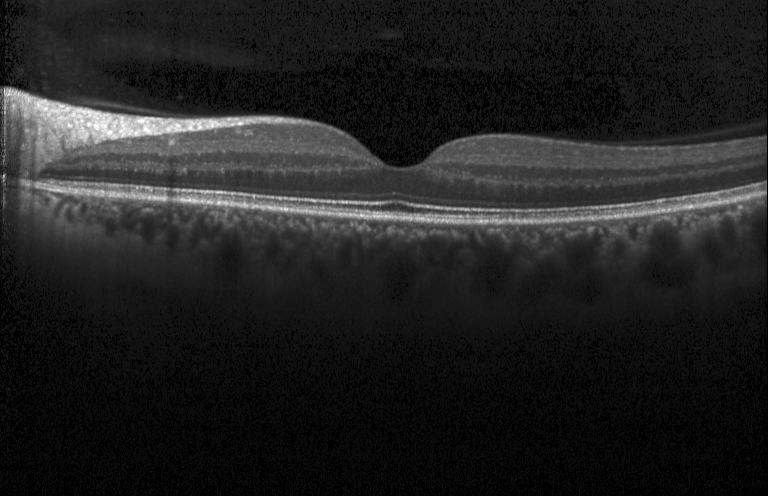 Retinal OCT B-scan
Impression: neither choroidal neovascularization, diabetic macular edema, nor drusen.